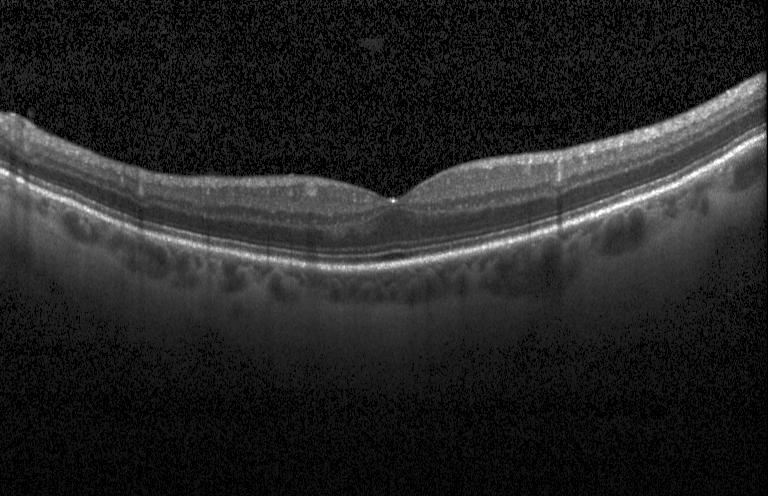

Retinal OCT cross-section; spectral-domain optical coherence tomography; centered on the fovea
Finding: no evidence of choroidal neovascularization, diabetic macular edema, or drusen.